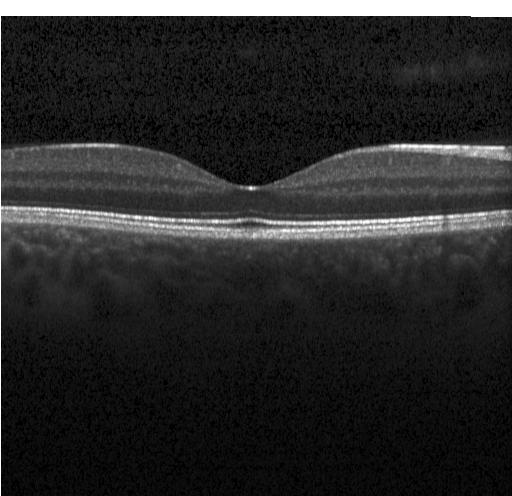
OCT finding: neither CNV, DME, nor drusen.